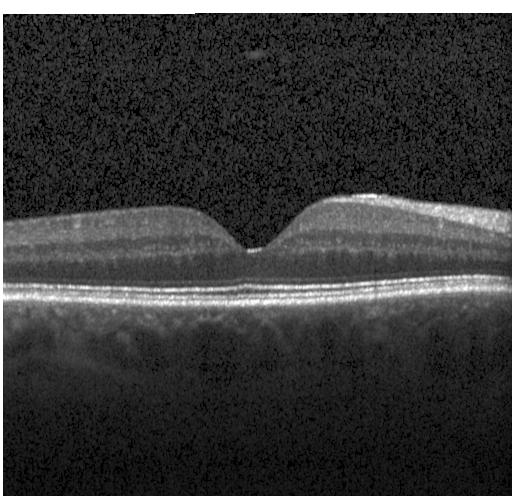
OCT B-scan · horizontal scan through the fovea — Neither choroidal neovascularization, diabetic macular edema, nor drusen.